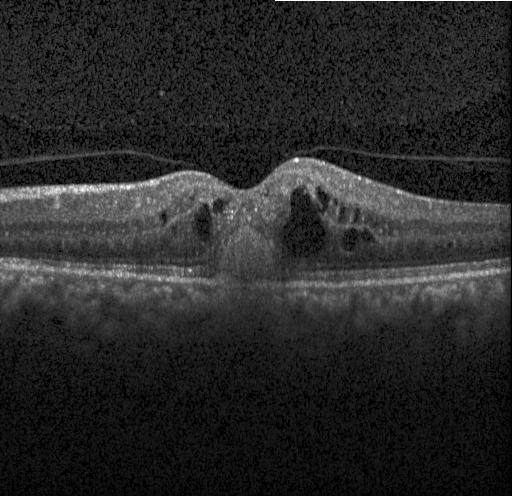

Macular OCT: CNV.